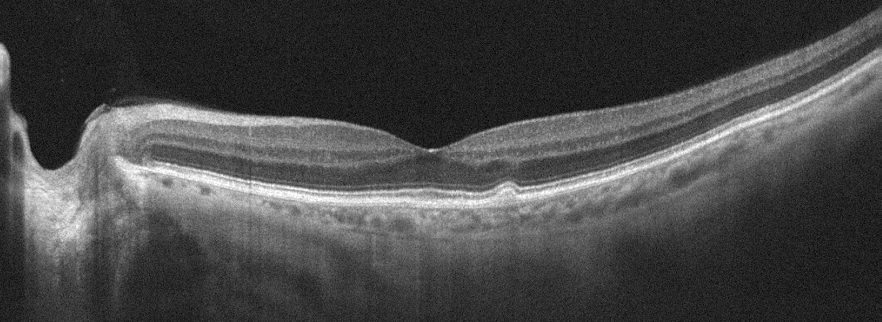 Oculus sinister. Optical coherence tomography B-scan
Finding: AMD.